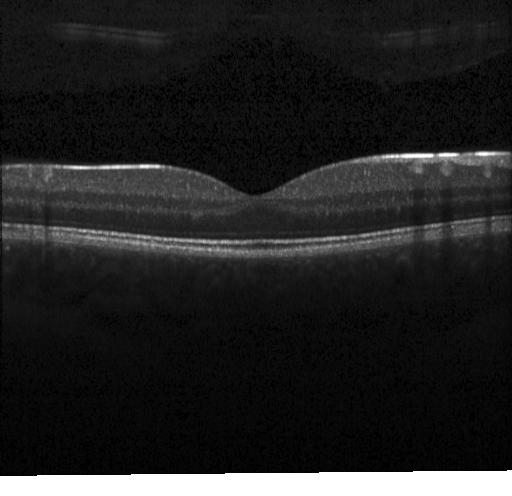
Instrument: Heidelberg Spectralis, optical coherence tomography scan. Macular OCT: neither choroidal neovascularization, diabetic macular edema, nor drusen.